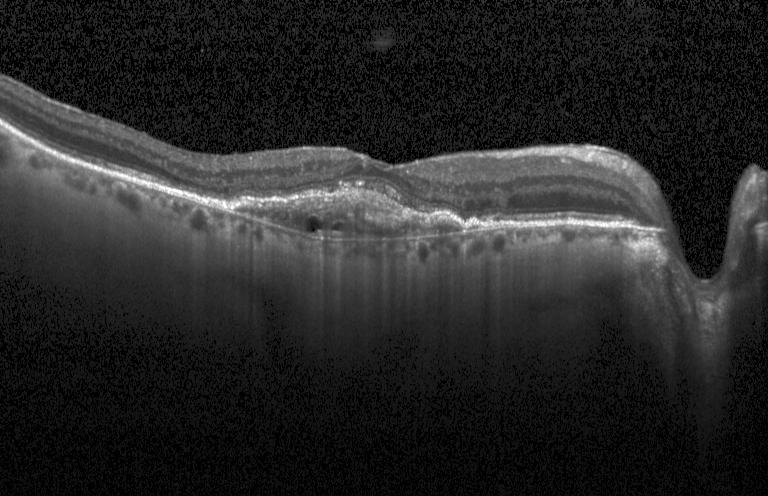

Instrument: Heidelberg Spectralis, retinal OCT cross-section — Assessment: choroidal neovascularization (CNV).